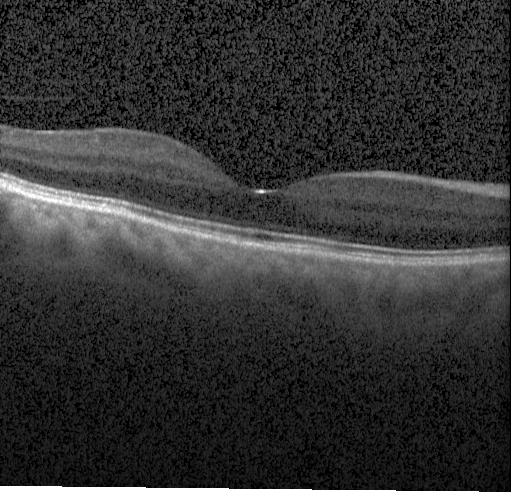

OCT line scan.
Impression: no choroidal neovascularization, diabetic macular edema, or drusen.